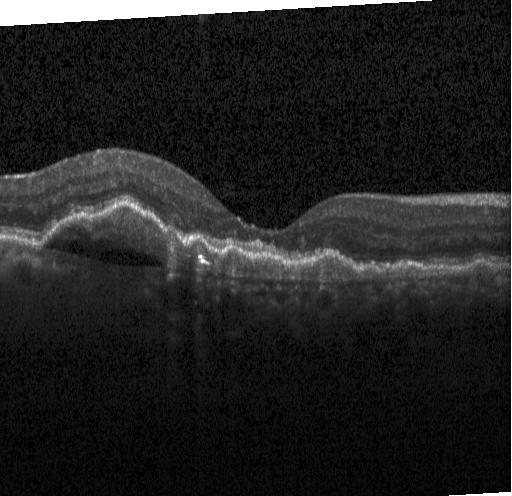

Impression: a choroidal neovascular membrane.